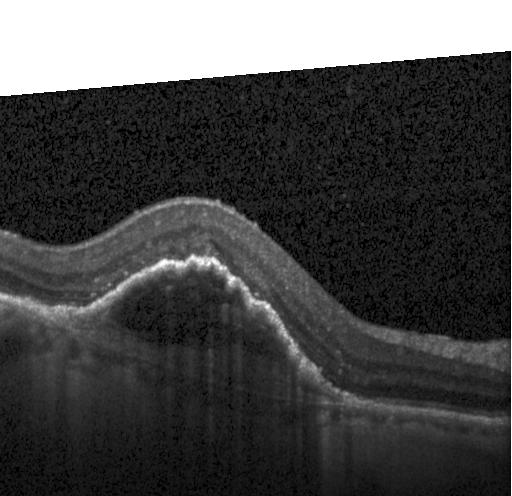

Macular OCT demonstrating CNV.